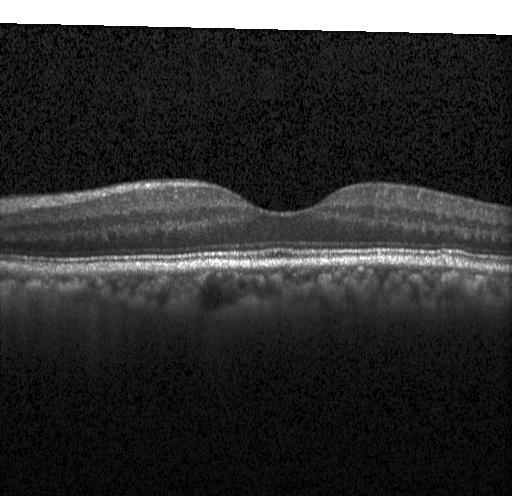 Retinal OCT B-scan
This B-scan demonstrates no choroidal neovascularization, diabetic macular edema, or drusen.